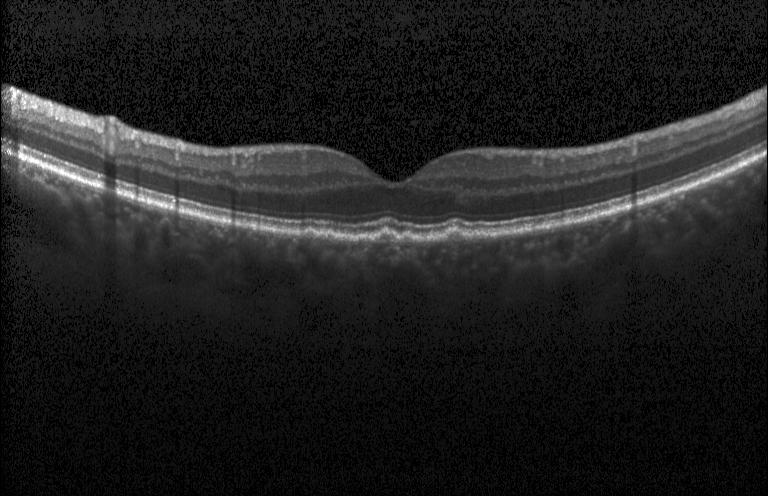

Retinal OCT cross-section, Heidelberg Spectralis.
Impression: multiple drusen.